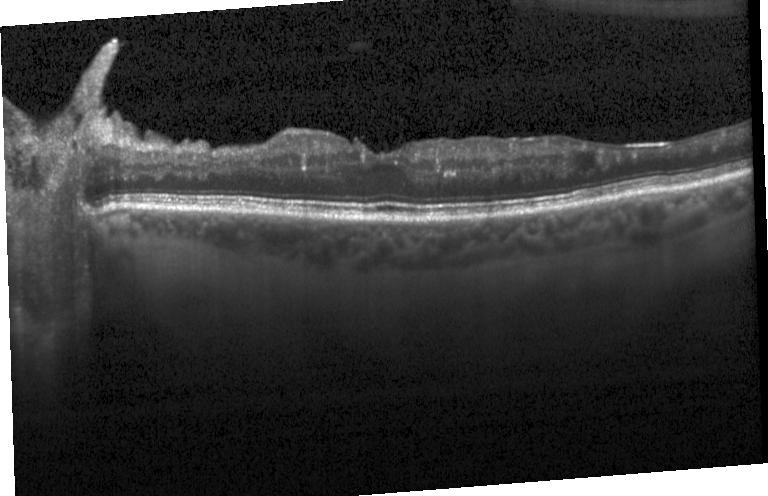

Spectral-domain OCT. Heidelberg Spectralis OCT system. Optical coherence tomography B-scan — Assessment: diabetic macular edema.